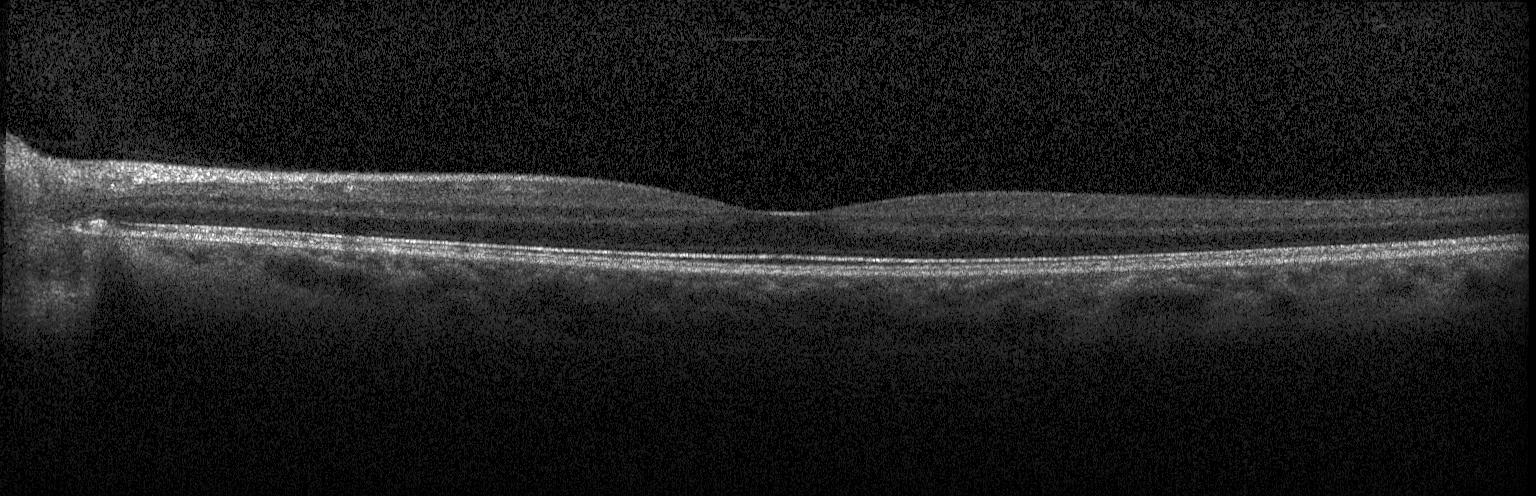

Centered on the fovea. Retinal OCT B-scan. Instrument: Heidelberg Spectralis. SD-OCT — Macular OCT: no choroidal neovascularization, no diabetic macular edema, and no drusen.